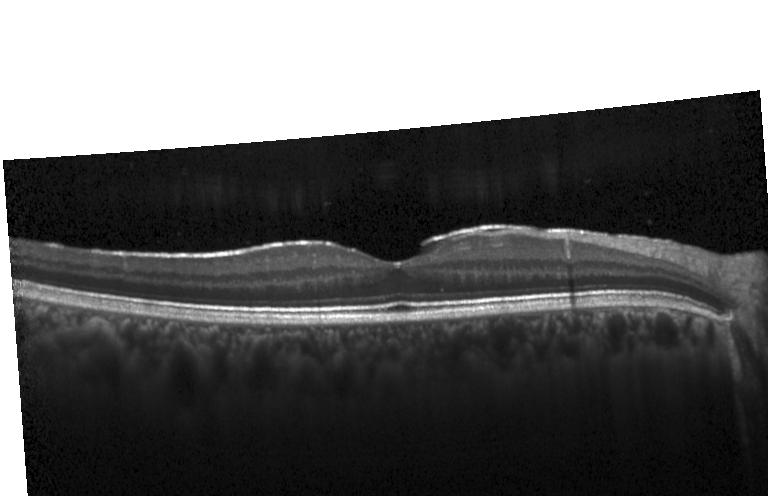

Optical coherence tomography B-scan. Macular OCT: neither choroidal neovascularization, diabetic macular edema, nor drusen.